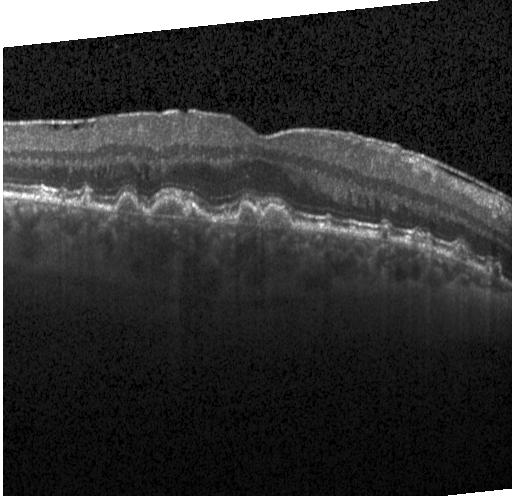 Diagnosis: multiple drusen.